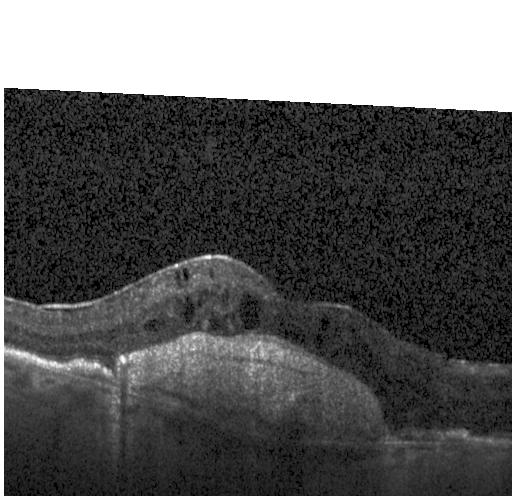 Heidelberg Spectralis, horizontal scan through the fovea, OCT B-scan, spectral-domain OCT. The scan shows a choroidal neovascular membrane.